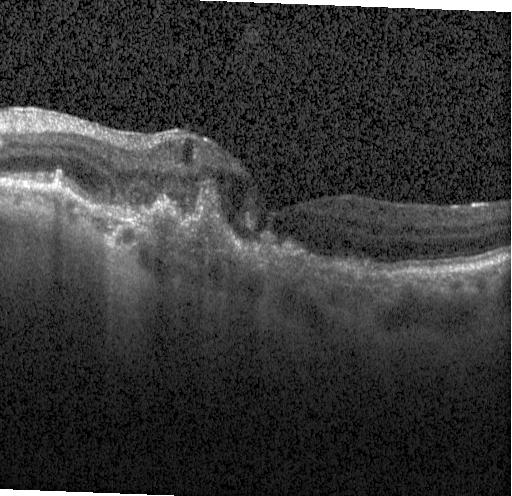

Fovea-centered; optical coherence tomography scan — Impression: a choroidal neovascular membrane.